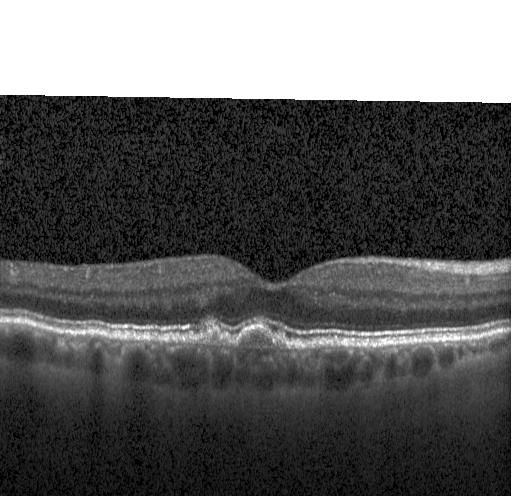 Optical coherence tomography scan; Heidelberg Spectralis OCT system; centered on the fovea — Impression: multiple drusen.